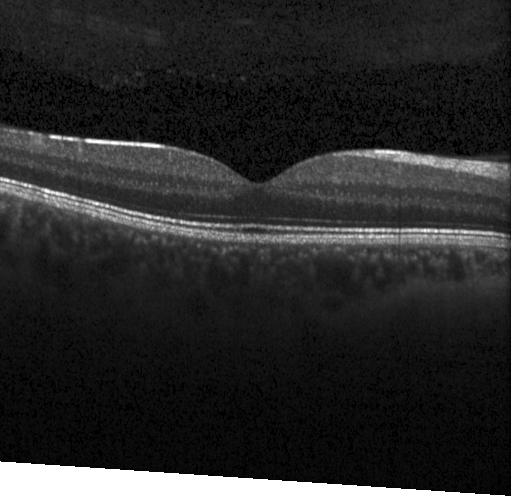

OCT B-scan showing no choroidal neovascularization, no diabetic macular edema, and no drusen.